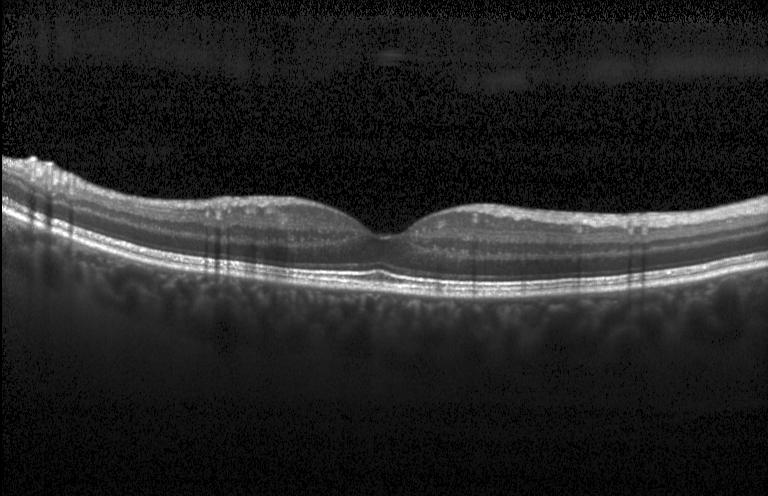 Diagnosis: no evidence of choroidal neovascularization, diabetic macular edema, or drusen.